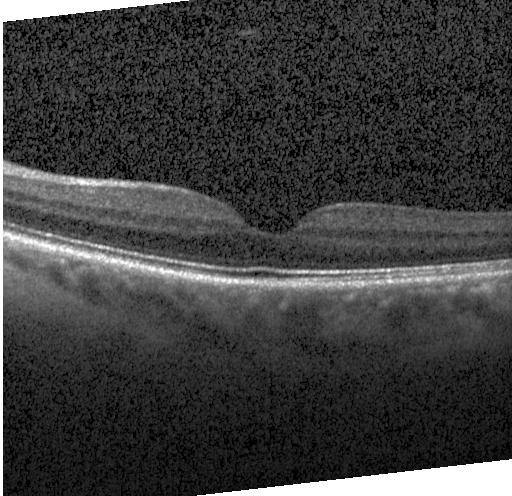
Retinal OCT B-scan. No evidence of CNV, DME, or drusen.